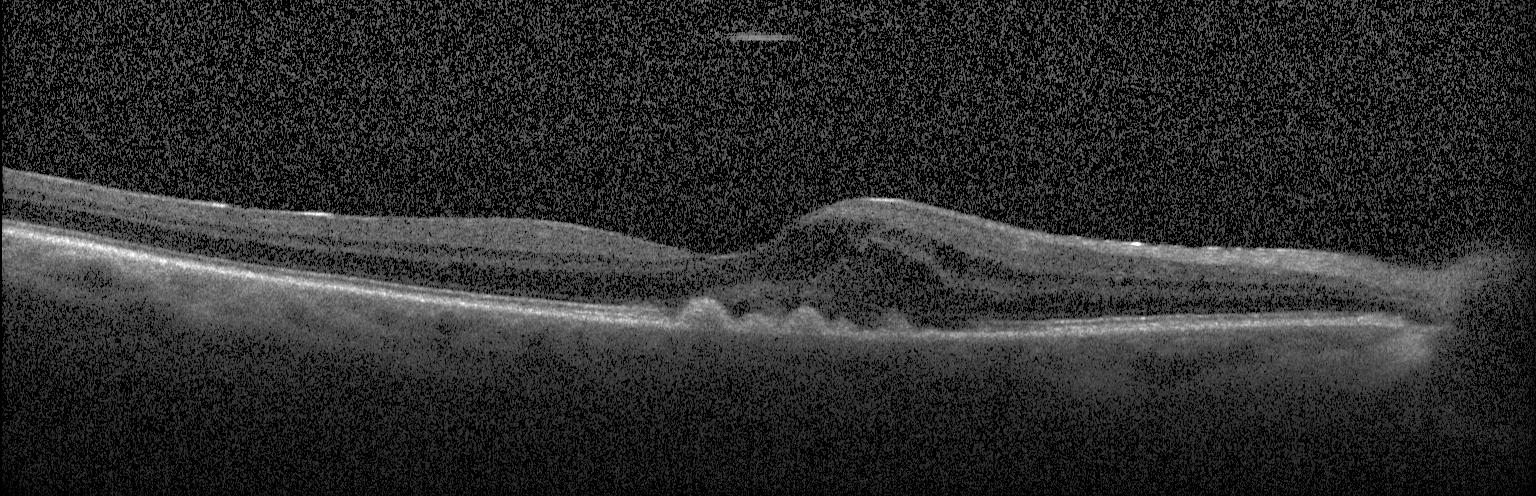

Spectral-domain optical coherence tomography. Acquired on a Heidelberg Spectralis. Optical coherence tomography B-scan.
Diagnosis: a choroidal neovascular membrane.